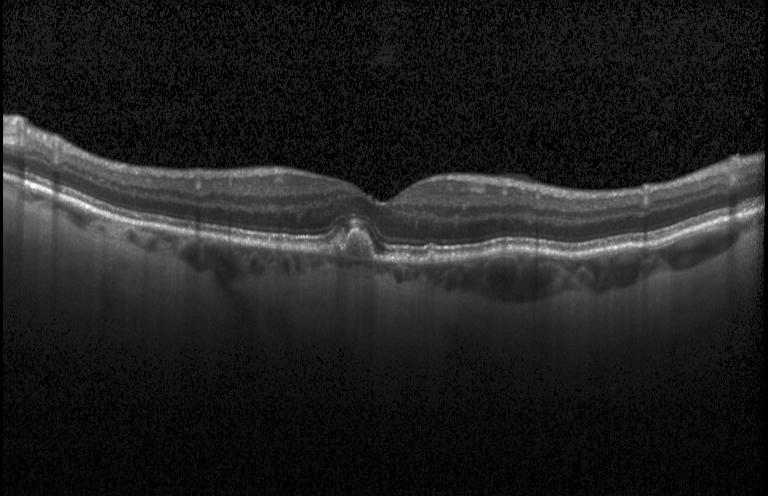
Assessment: sub-RPE drusenoid deposits.